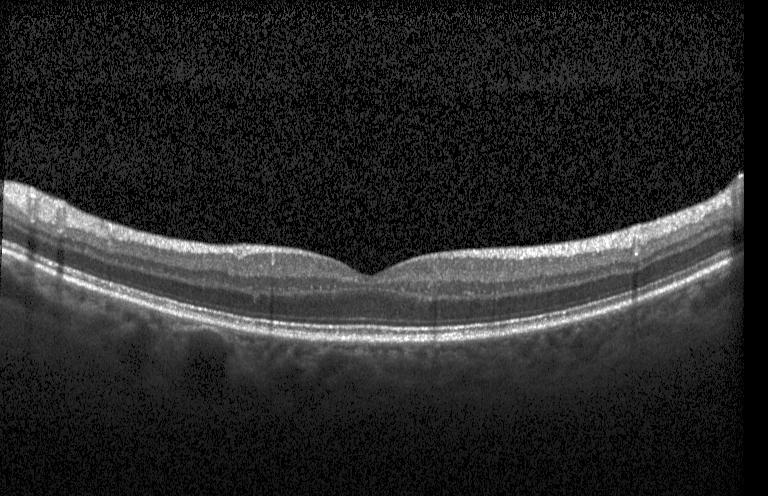
This B-scan demonstrates no evidence of CNV, DME, or drusen.